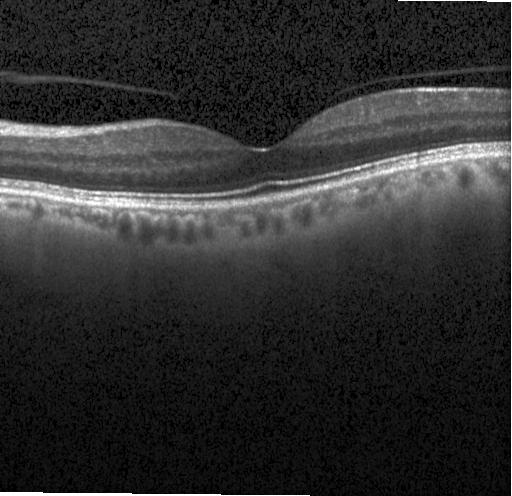
OCT line scan
Finding: no evidence of choroidal neovascularization, diabetic macular edema, or drusen.